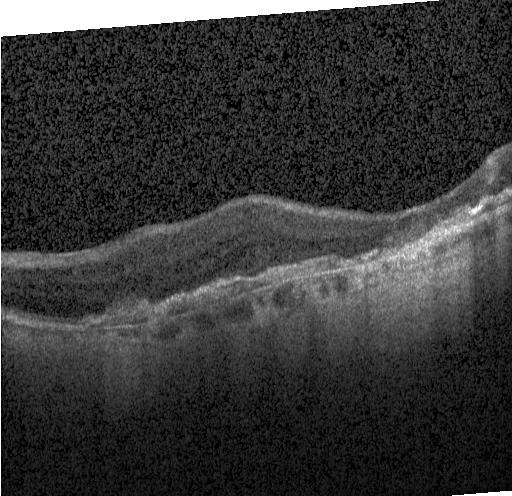 Retinal OCT cross-section, SD-OCT. Impression: a choroidal neovascular membrane.